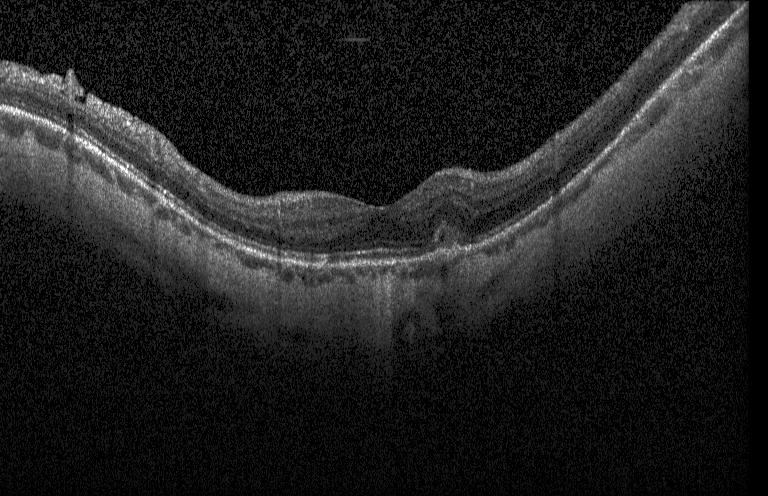 Retinal OCT B-scan.
Impression: a choroidal neovascular membrane.